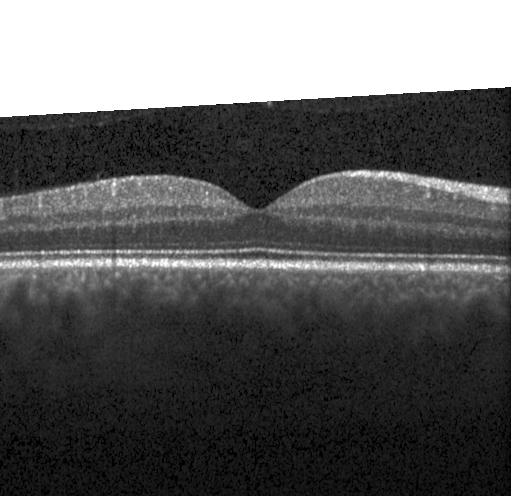 Retinal OCT B-scan; spectral-domain OCT; fovea-centered. Assessment: neither choroidal neovascularization, diabetic macular edema, nor drusen.